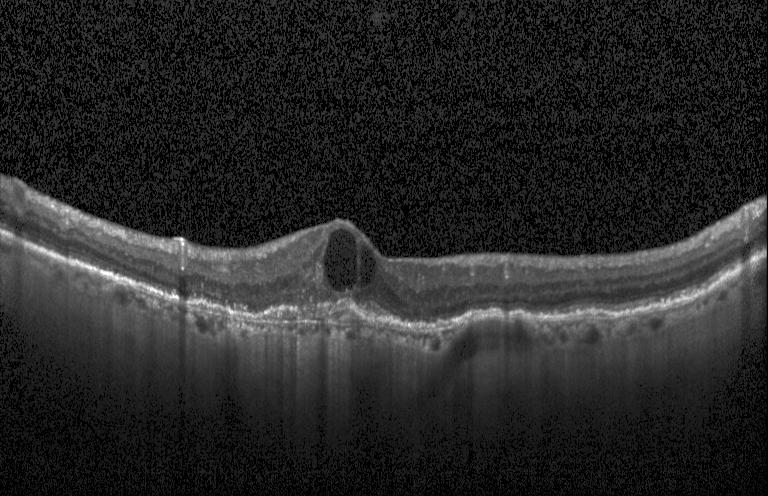 Impression: choroidal neovascularization.